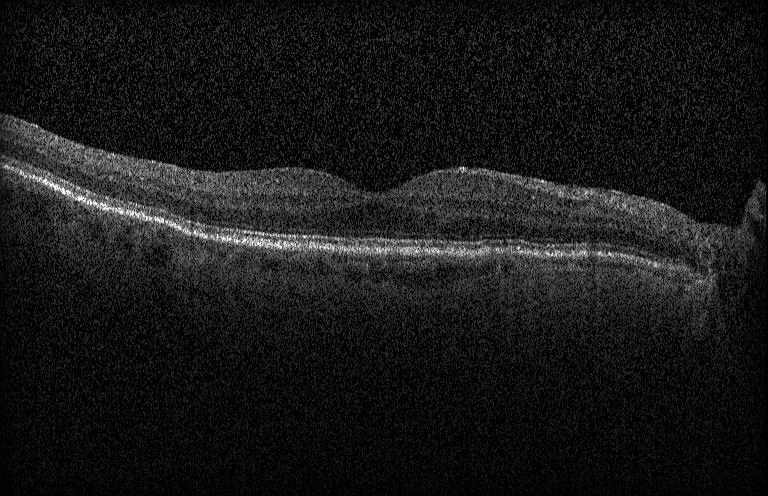

Macular OCT demonstrating no choroidal neovascularization, no diabetic macular edema, and no drusen.